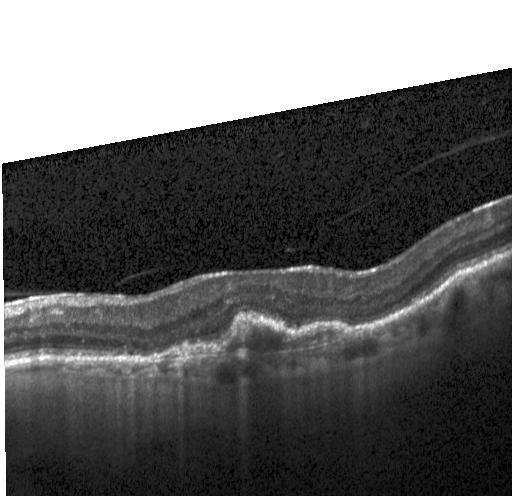

OCT scan showing a choroidal neovascular membrane.